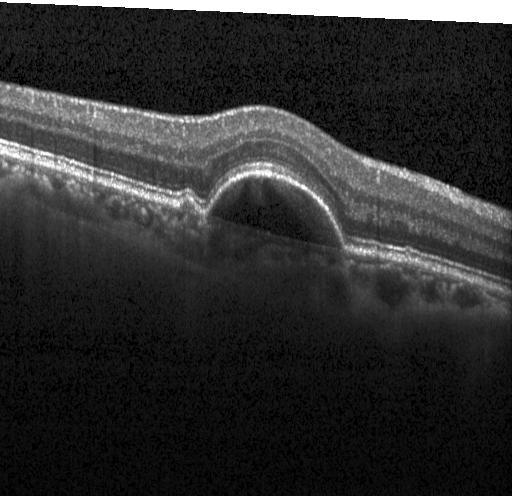

OCT scan showing choroidal neovascularization.